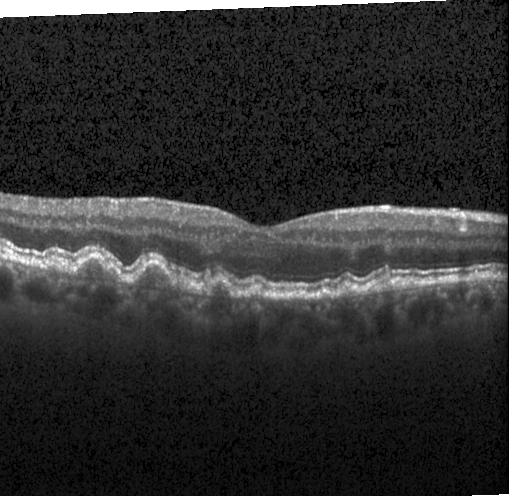
Heidelberg Spectralis; optical coherence tomography scan; spectral-domain OCT
Impression: drusen.